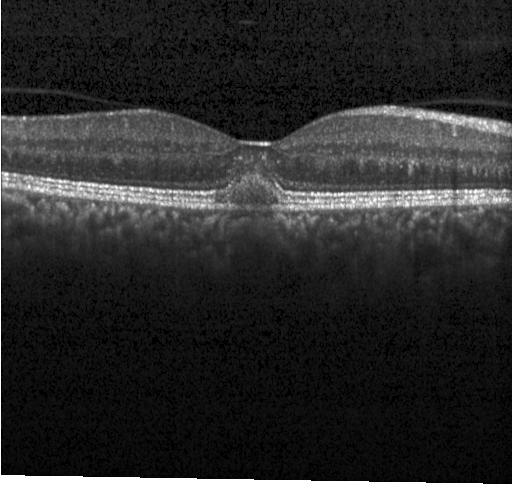
OCT B-scan — Choroidal neovascularization.